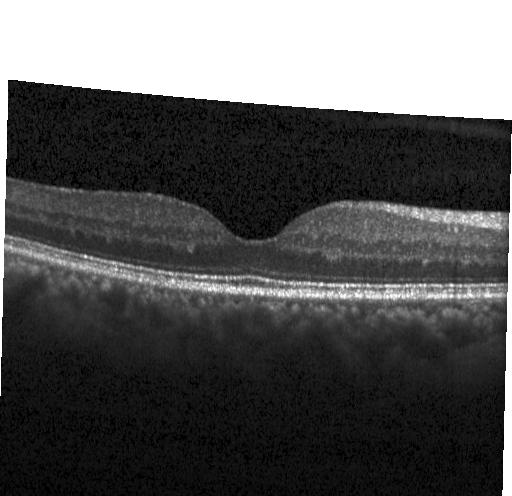 Optical coherence tomography B-scan; spectral-domain optical coherence tomography; instrument: Heidelberg Spectralis.
The scan shows no choroidal neovascularization, diabetic macular edema, or drusen.